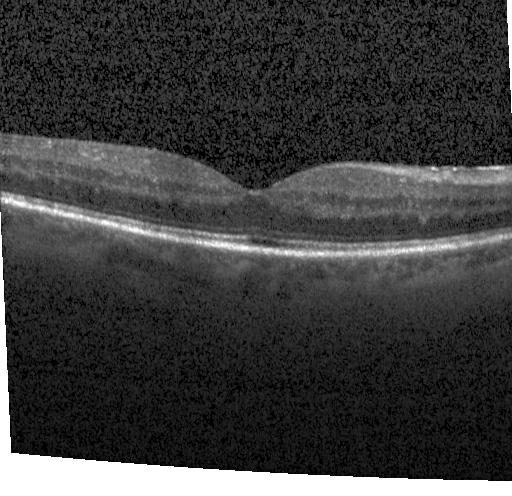

Spectral-domain OCT B-scan: no choroidal neovascularization, diabetic macular edema, or drusen.